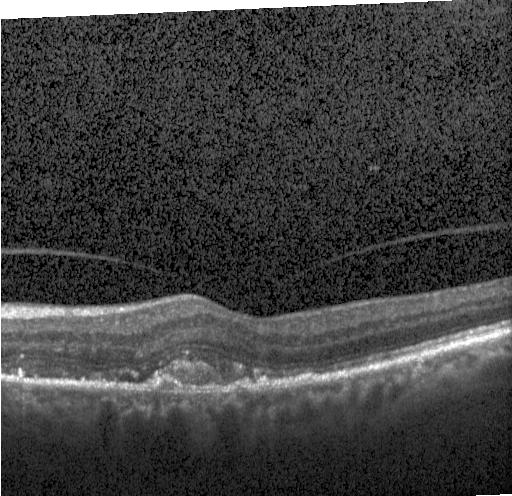

Optical coherence tomography B-scan. This B-scan demonstrates choroidal neovascularization (CNV).